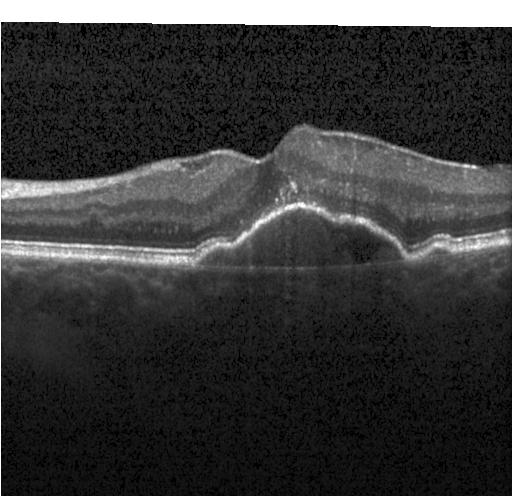

Spectral-domain optical coherence tomography; OCT line scan. Finding: choroidal neovascularization.